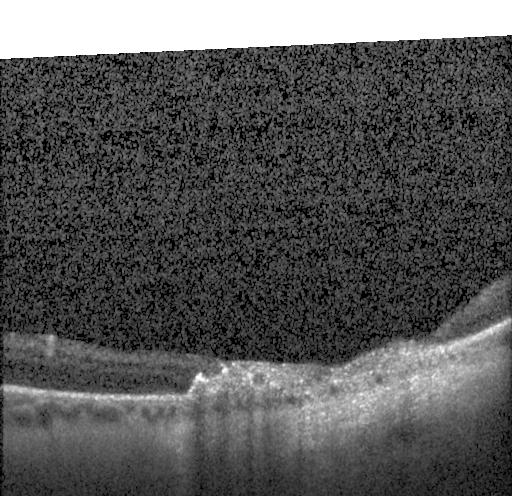
Spectral-domain optical coherence tomography; retinal OCT cross-section; acquired on a Heidelberg Spectralis — Dx: choroidal neovascularization (CNV).